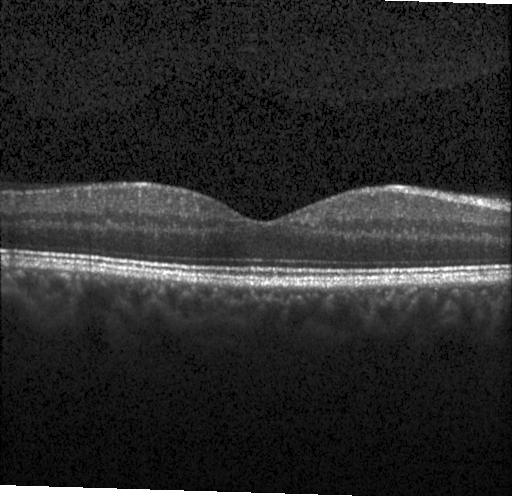

Diagnosis: no evidence of CNV, DME, or drusen.